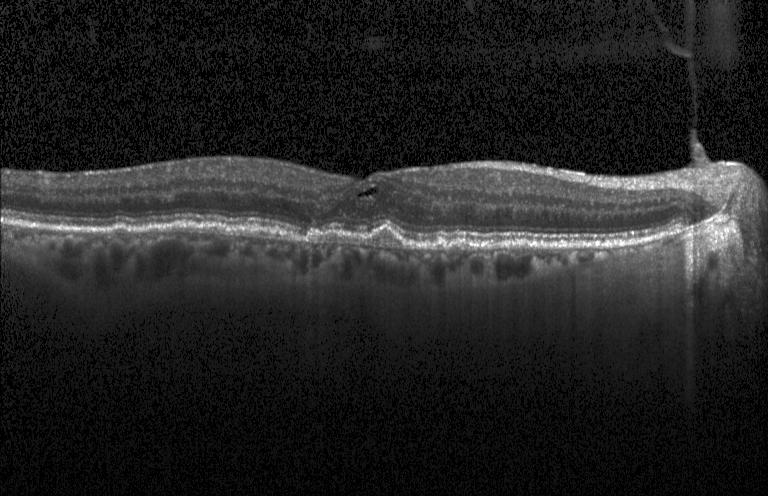

SD-OCT. Instrument: Heidelberg Spectralis. Through the macula. OCT B-scan — Diagnosis: CNV.